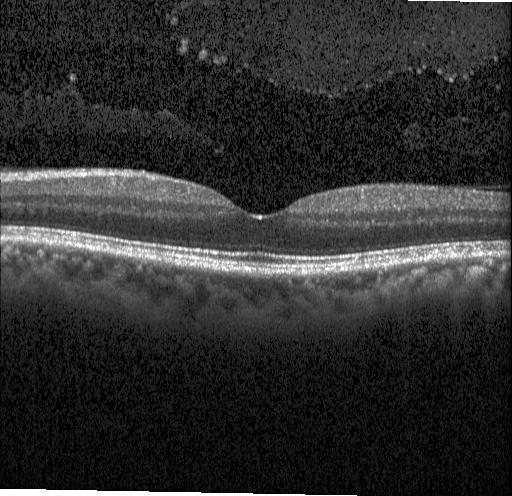

Optical coherence tomography B-scan. Finding: no choroidal neovascularization, no diabetic macular edema, and no drusen.